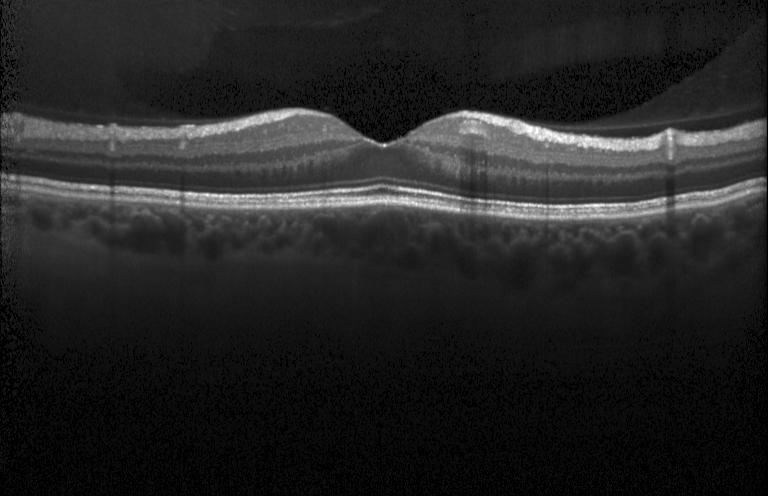

OCT scan showing no CNV, DME, or drusen.